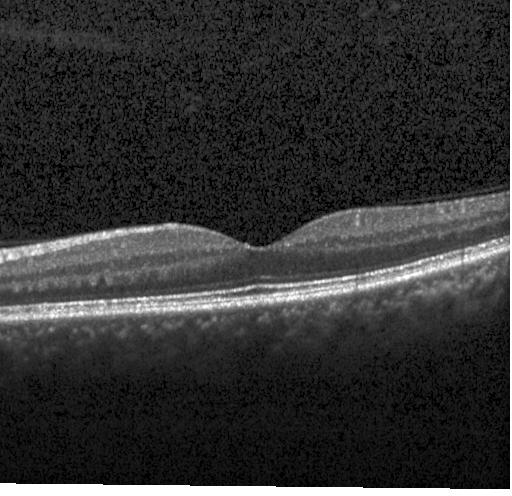

OCT finding: neither CNV, DME, nor drusen.